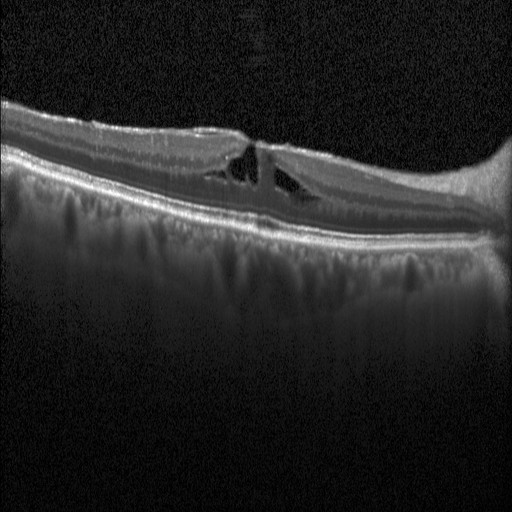 Spectral-domain OCT · centered on the fovea · OCT B-scan · acquired on a Heidelberg Spectralis — This B-scan demonstrates DME.